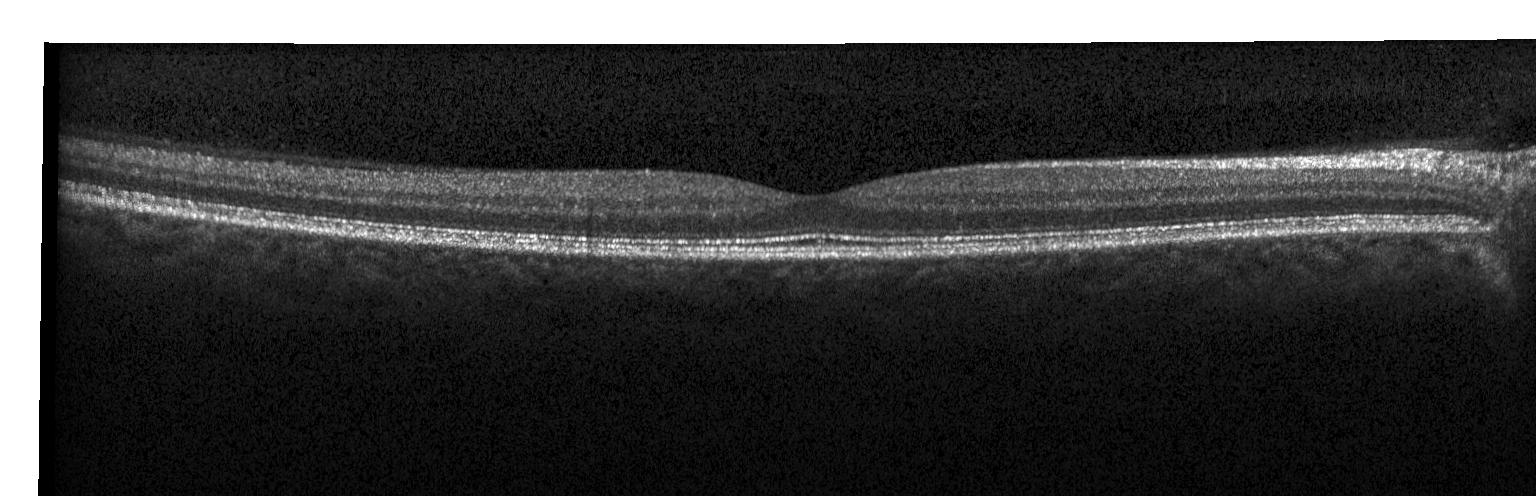

Assessment: no CNV, DME, or drusen.